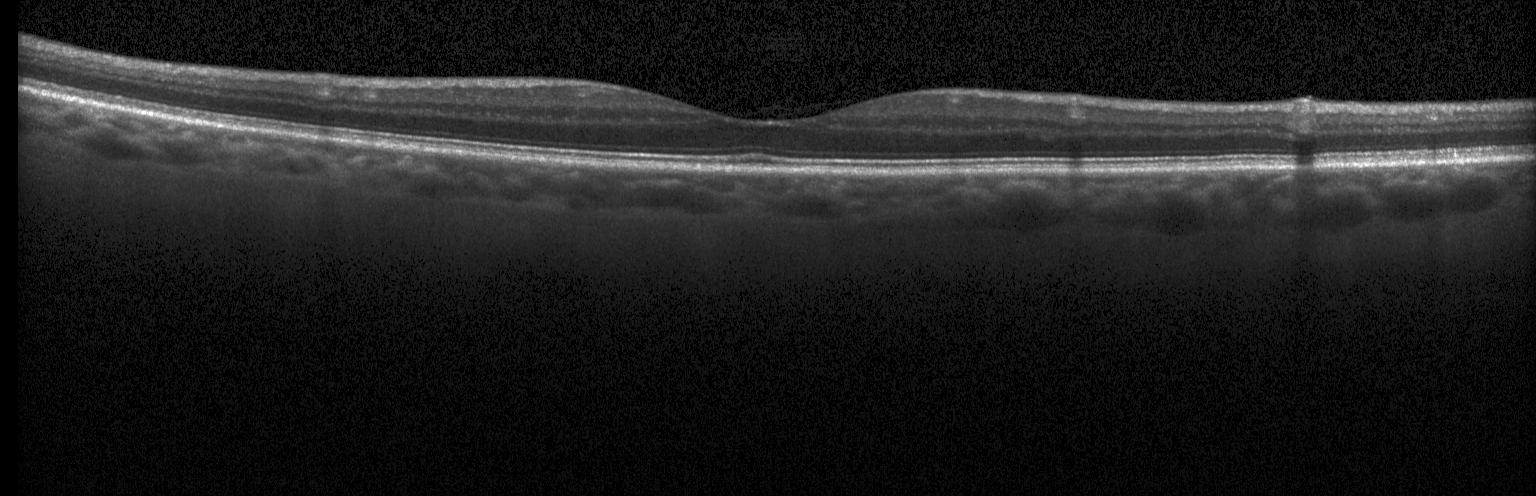

Heidelberg Spectralis · SD-OCT · through the macula · optical coherence tomography scan
Impression: no choroidal neovascularization, no diabetic macular edema, and no drusen.